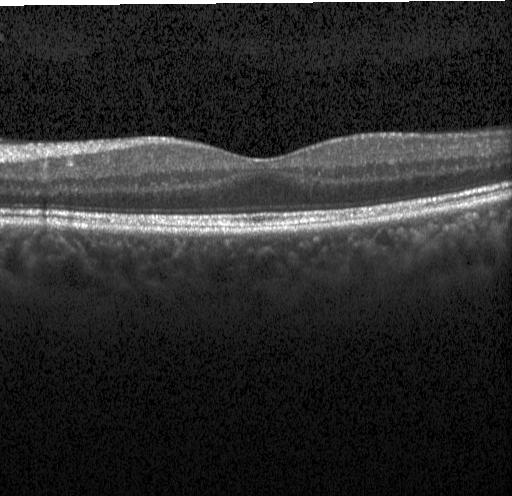

OCT line scan; macular scan.
Macular OCT: no evidence of choroidal neovascularization, diabetic macular edema, or drusen.